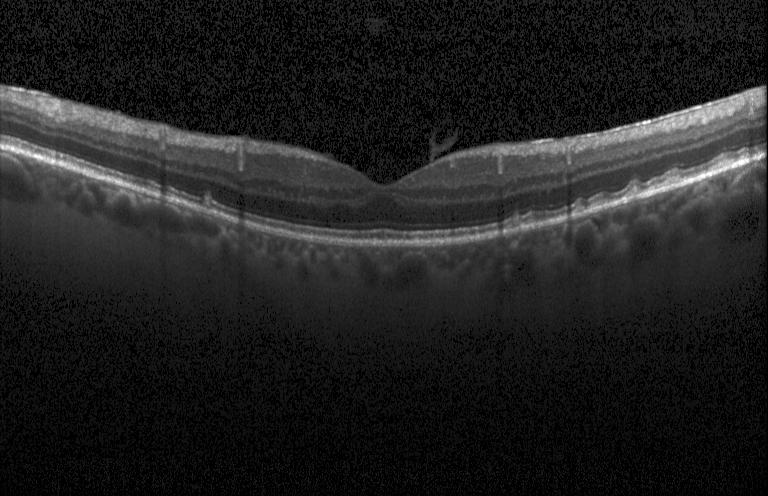
The scan shows multiple drusen.